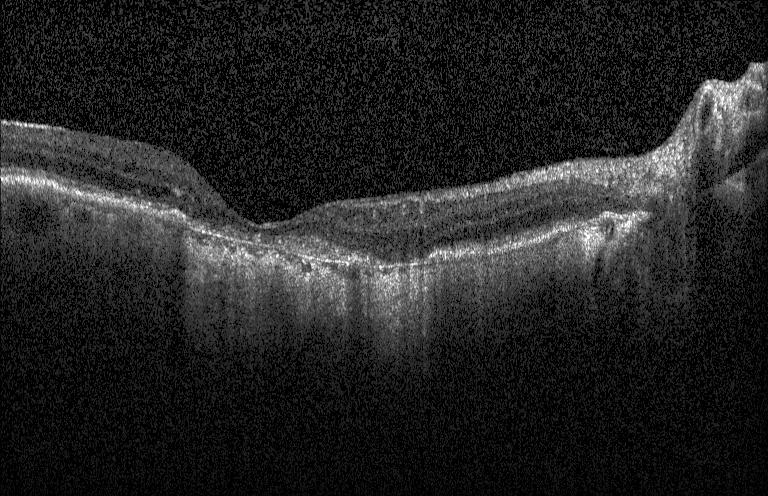

Spectral-domain optical coherence tomography. Optical coherence tomography B-scan — Finding: CNV.